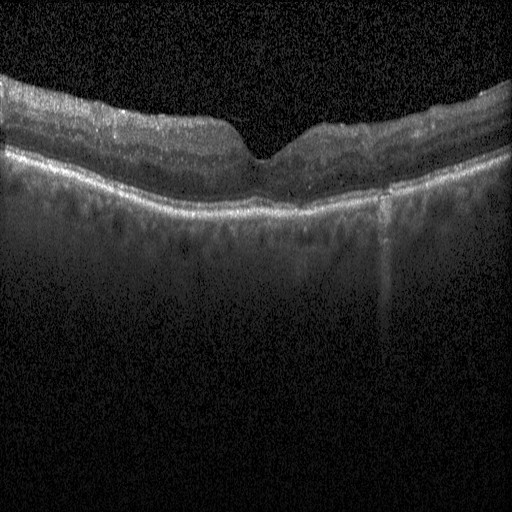
Retinal OCT B-scan; spectral-domain optical coherence tomography; Heidelberg Spectralis OCT system — OCT finding: diabetic macular edema (DME).